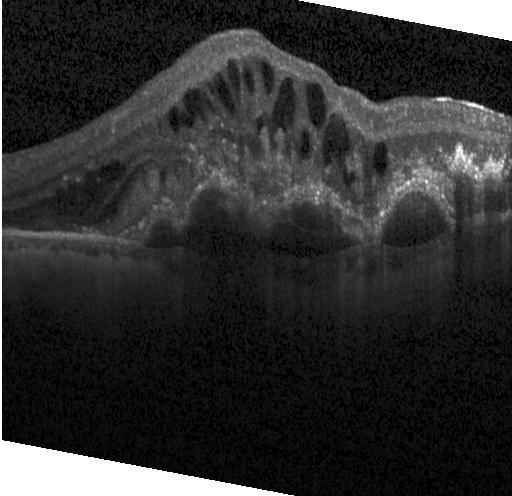

OCT B-scan; SD-OCT; horizontal scan through the fovea; Heidelberg Spectralis OCT system — This B-scan demonstrates a choroidal neovascular membrane.